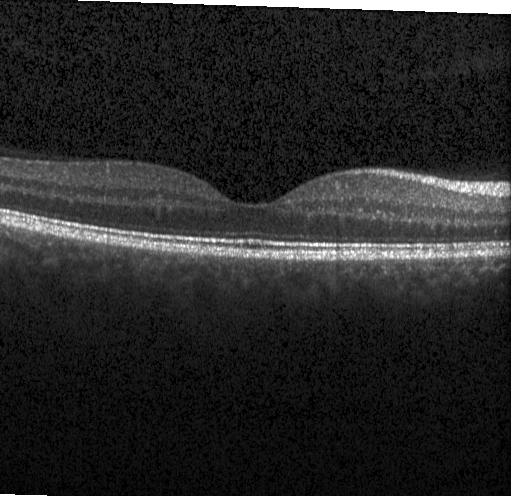 Impression: neither choroidal neovascularization, diabetic macular edema, nor drusen.